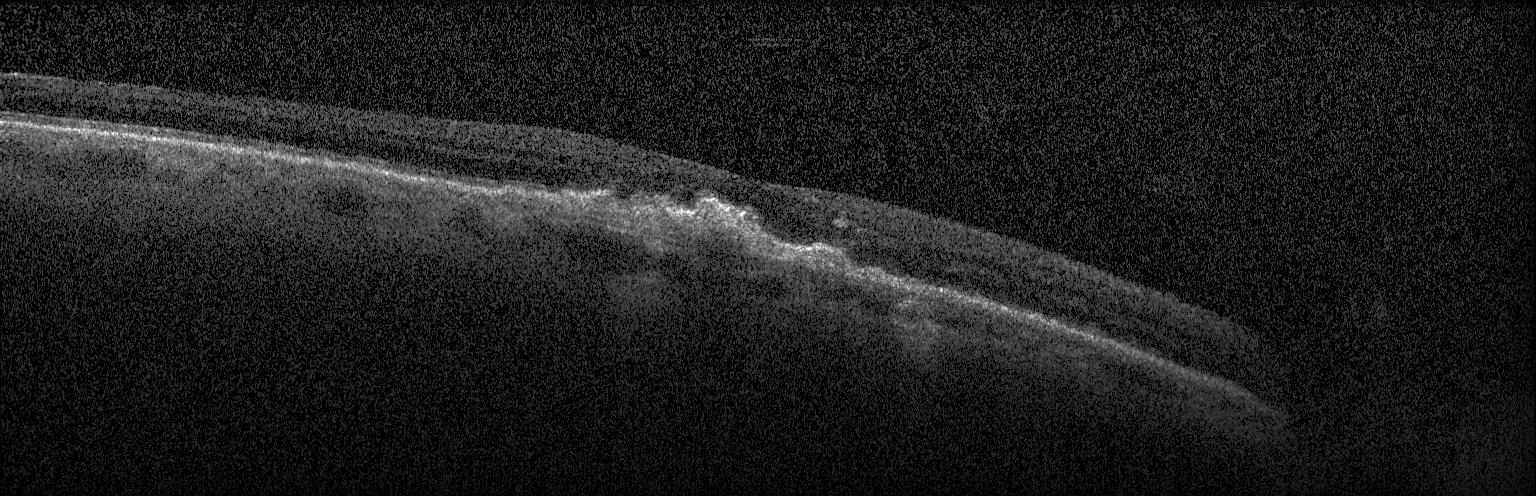 This B-scan demonstrates CNV.